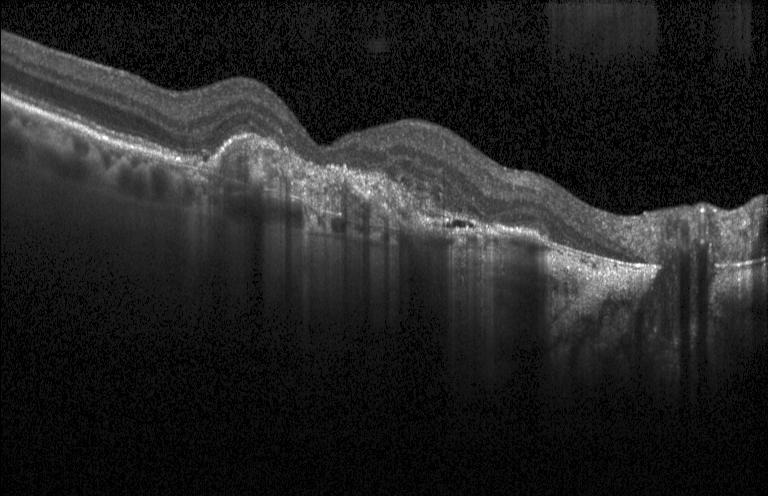

Finding: a choroidal neovascular membrane.